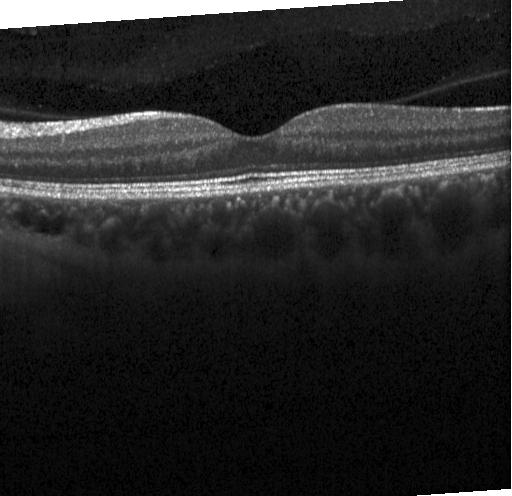
Acquired on a Heidelberg Spectralis; OCT B-scan; horizontal scan through the fovea — Finding: neither choroidal neovascularization, diabetic macular edema, nor drusen.